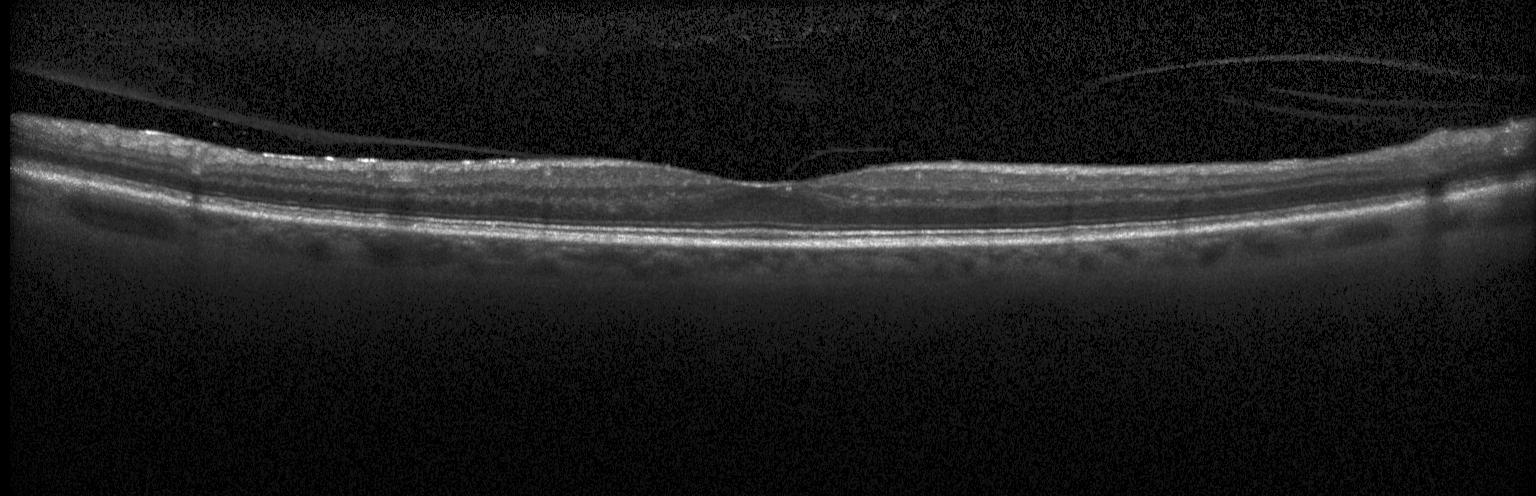 Spectral-domain OCT; optical coherence tomography scan. Assessment: no choroidal neovascularization, diabetic macular edema, or drusen.